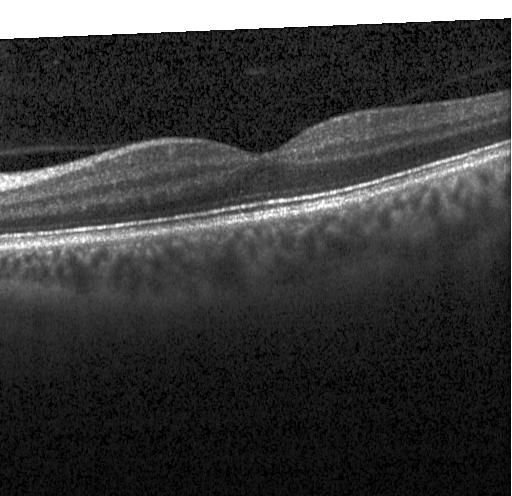

Impression: no CNV, no DME, and no drusen.